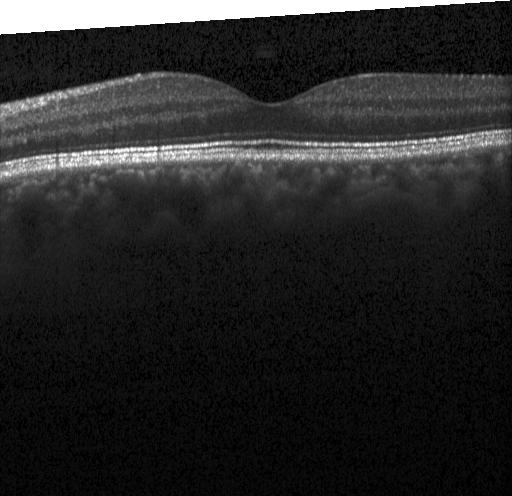 Acquired on a Heidelberg Spectralis · centered on the fovea · retinal OCT cross-section · SD-OCT — Diagnosis: no choroidal neovascularization, diabetic macular edema, or drusen.